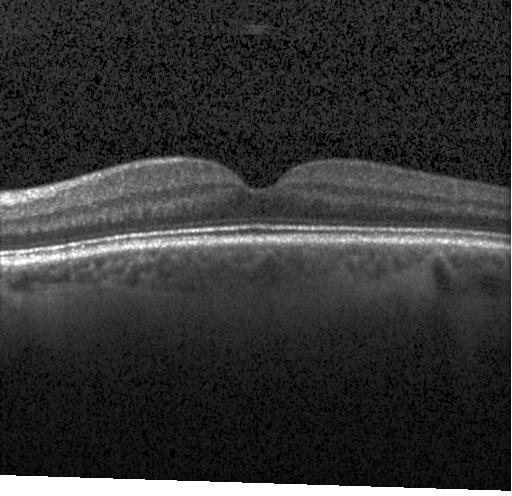 OCT finding: no evidence of choroidal neovascularization, diabetic macular edema, or drusen.